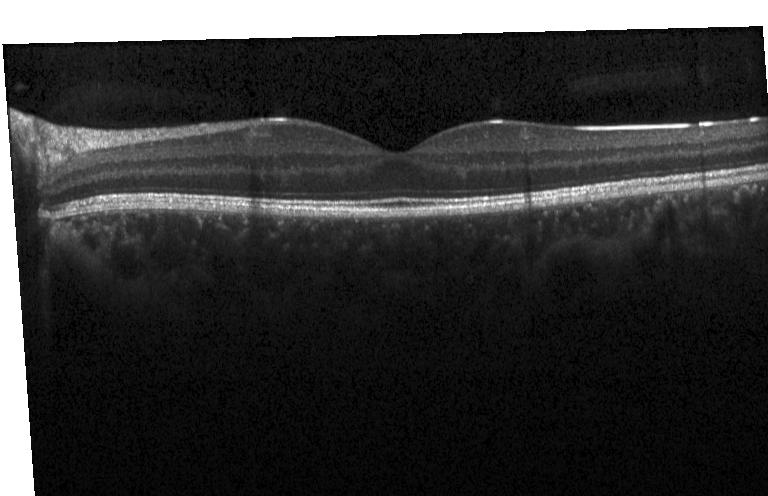
OCT line scan. Macular scan. No CNV, no DME, and no drusen.